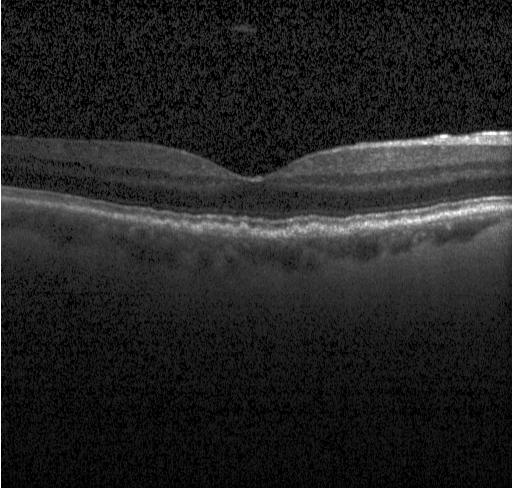
Impression: sub-RPE drusenoid deposits.